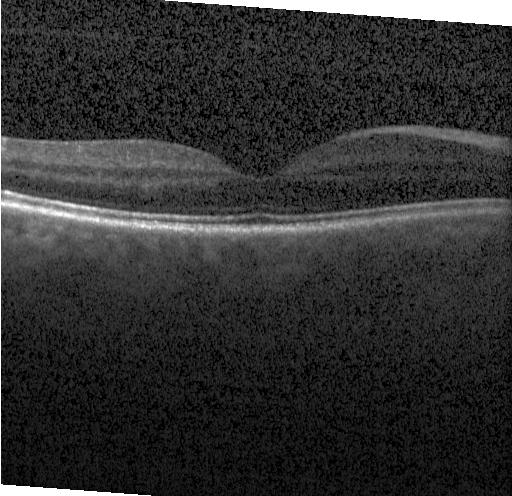 Acquired on a Heidelberg Spectralis · macular scan · spectral-domain OCT · OCT B-scan.
Macular OCT: neither choroidal neovascularization, diabetic macular edema, nor drusen.